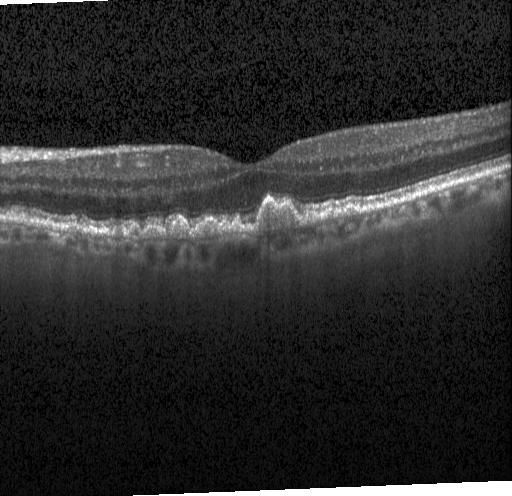
Macular OCT: sub-RPE drusenoid deposits.